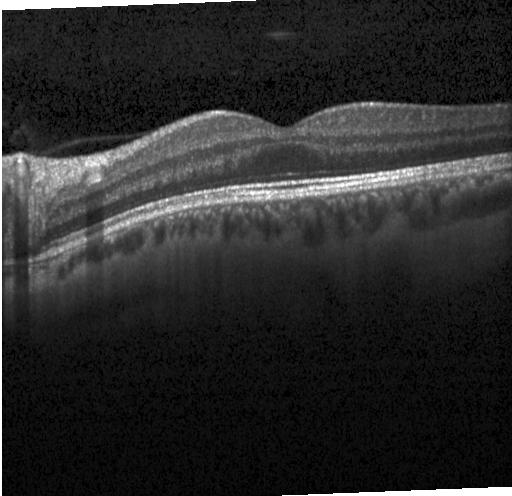 Optical coherence tomography B-scan. Macular scan.
No evidence of choroidal neovascularization, diabetic macular edema, or drusen.